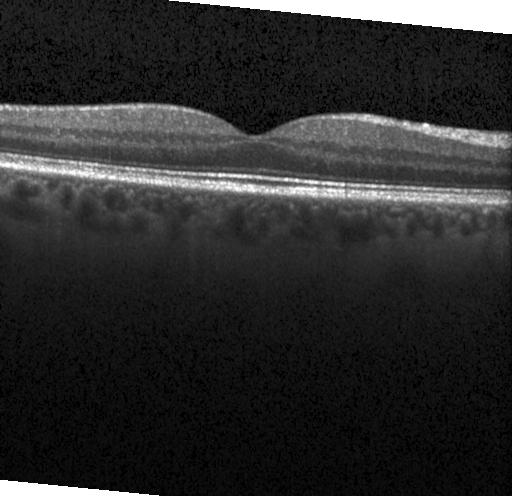

Optical coherence tomography B-scan, through the macula.
No evidence of choroidal neovascularization, diabetic macular edema, or drusen.